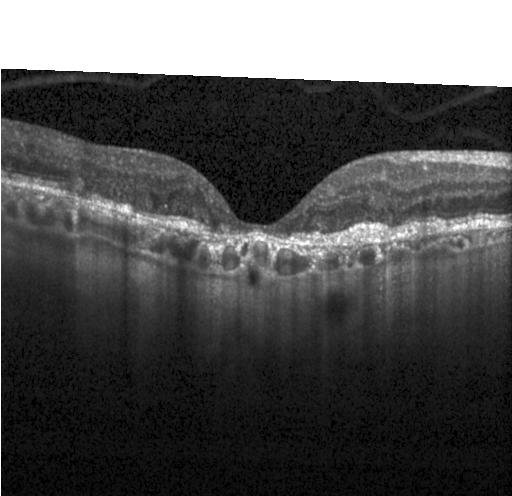

OCT B-scan; Heidelberg Spectralis
OCT finding: choroidal neovascularization (CNV).